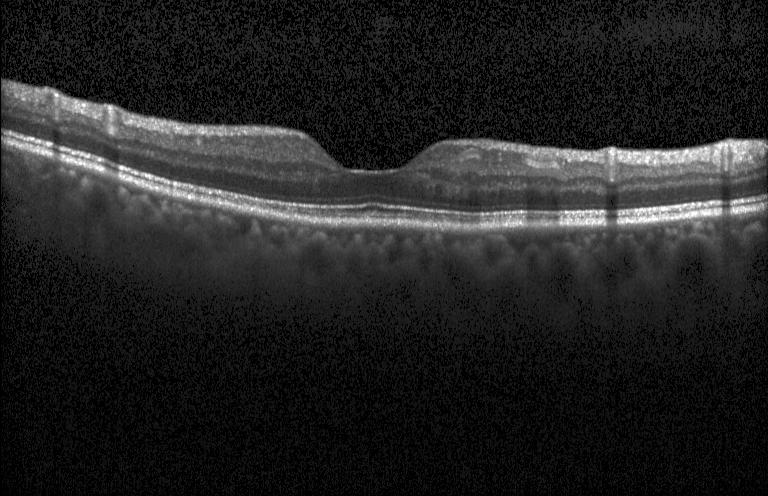

Horizontal scan through the fovea; retinal OCT cross-section
No choroidal neovascularization, diabetic macular edema, or drusen.